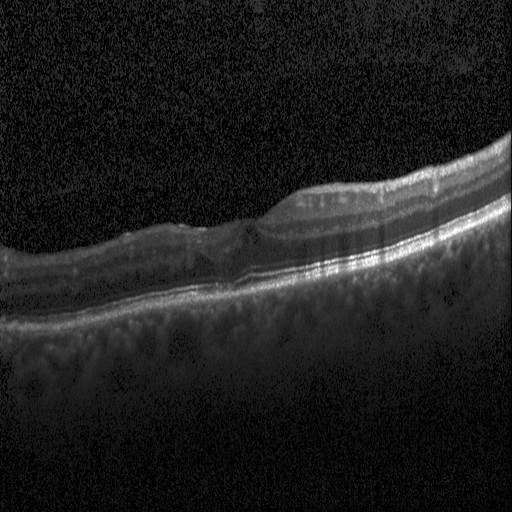
Heidelberg Spectralis · centered on the fovea · retinal OCT B-scan · spectral-domain optical coherence tomography.
OCT finding: DME.